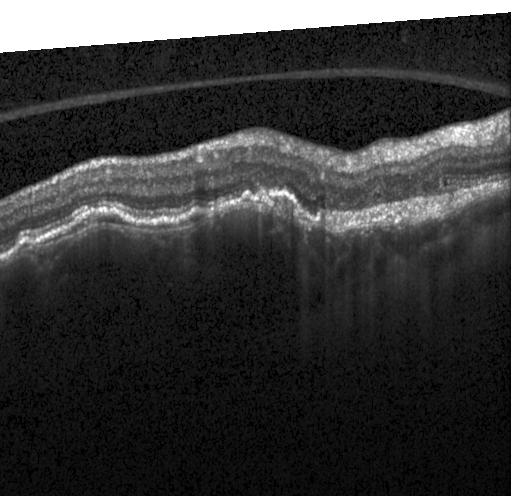
Retinal OCT B-scan
Impression: a choroidal neovascular membrane.